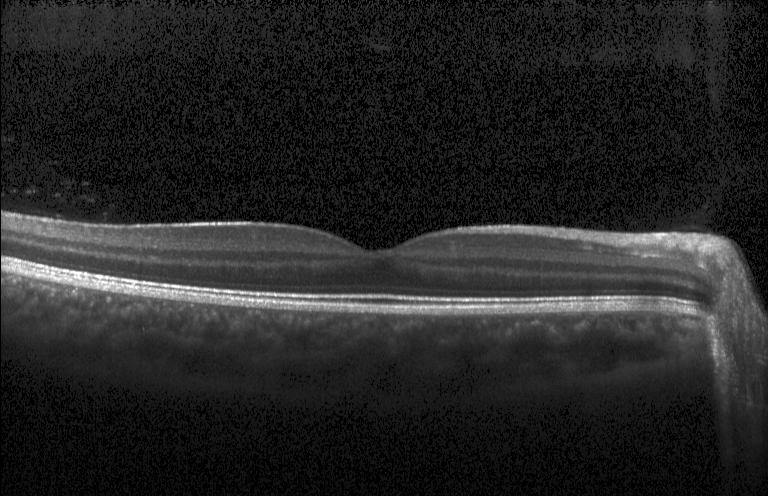
Instrument: Heidelberg Spectralis; spectral-domain OCT; OCT B-scan; horizontal scan through the fovea — OCT finding: no evidence of choroidal neovascularization, diabetic macular edema, or drusen.